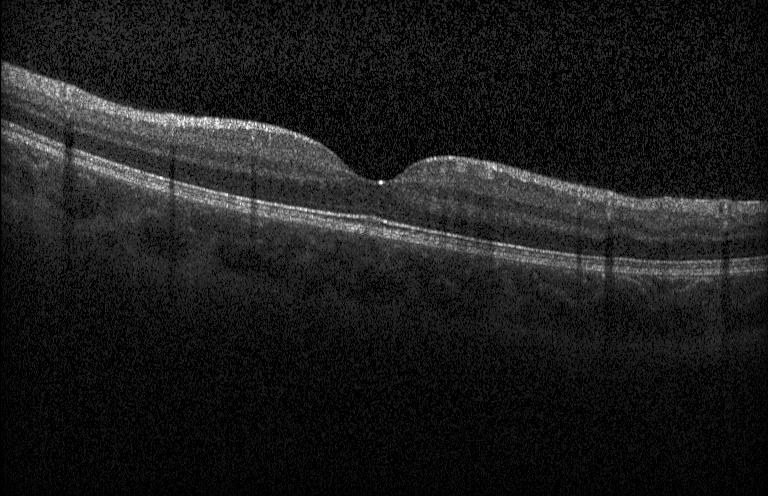
Optical coherence tomography scan
Impression: neither choroidal neovascularization, diabetic macular edema, nor drusen.